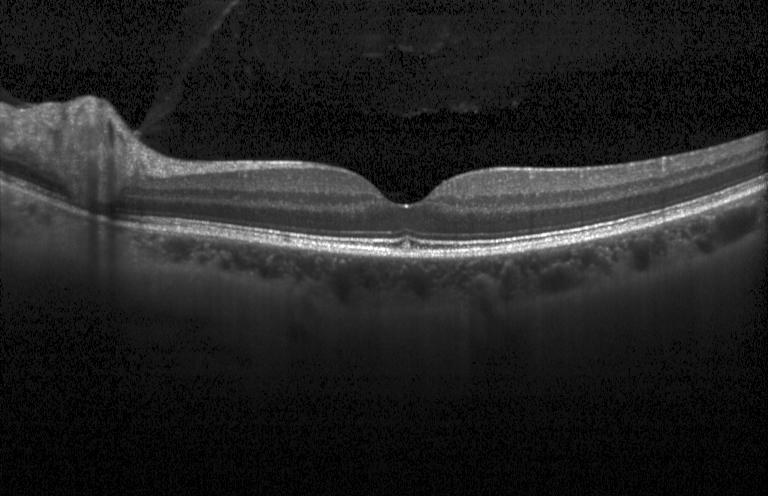

Assessment: no evidence of CNV, DME, or drusen.